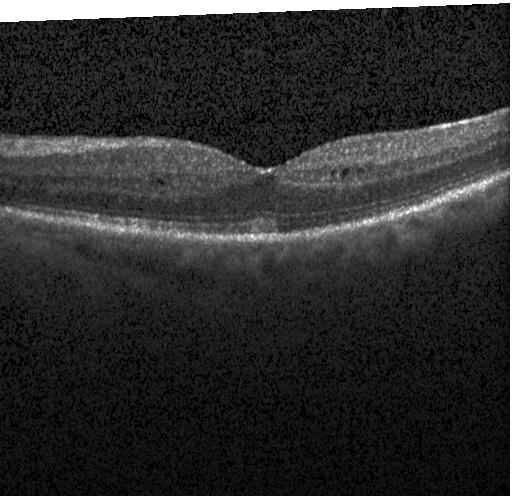

OCT line scan. Through the macula. Acquired on a Heidelberg Spectralis. Impression: DME.